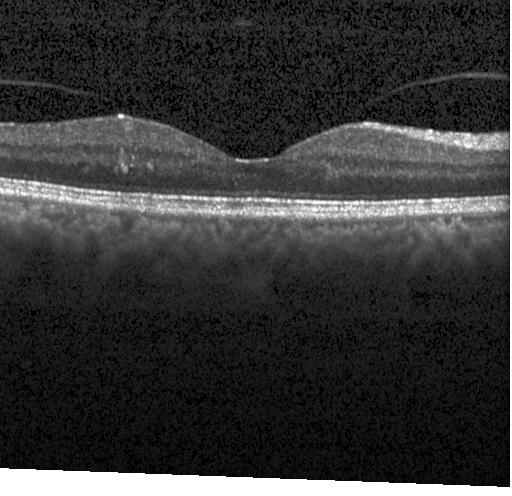 Assessment: neither choroidal neovascularization, diabetic macular edema, nor drusen.